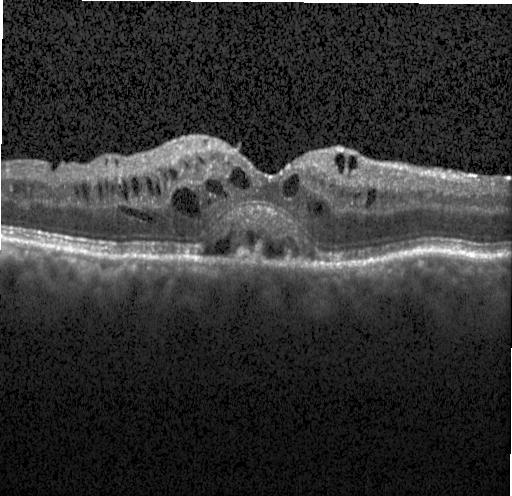 Spectral-domain OCT · OCT B-scan · Heidelberg Spectralis. Finding: DME.